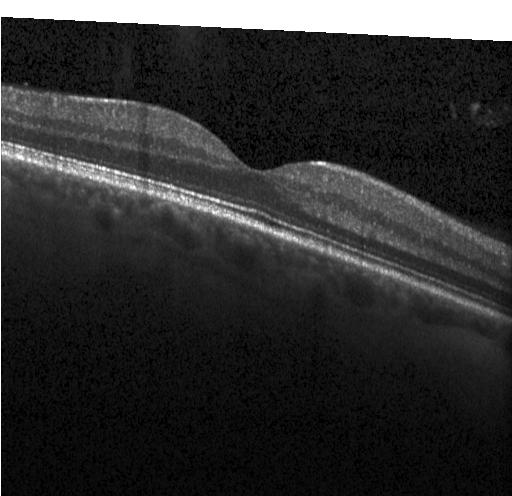 Through the macula; spectral-domain OCT; instrument: Heidelberg Spectralis; optical coherence tomography B-scan
Impression: no CNV, no DME, and no drusen.